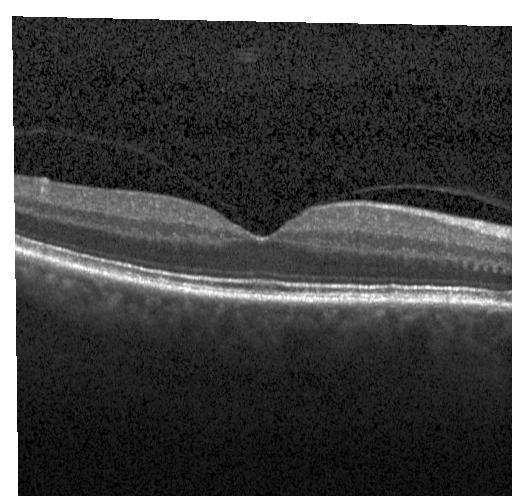
Optical coherence tomography B-scan, through the macula — Diagnosis: no choroidal neovascularization, diabetic macular edema, or drusen.